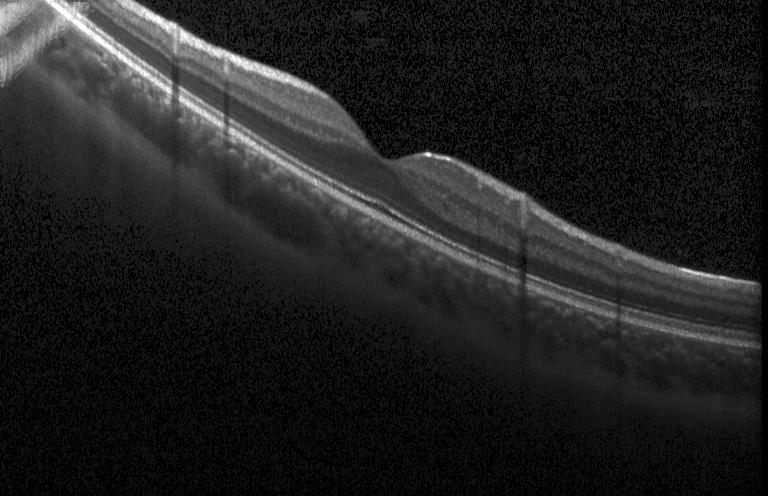
Optical coherence tomography scan · spectral-domain optical coherence tomography · instrument: Heidelberg Spectralis · centered on the fovea
No evidence of choroidal neovascularization, diabetic macular edema, or drusen.